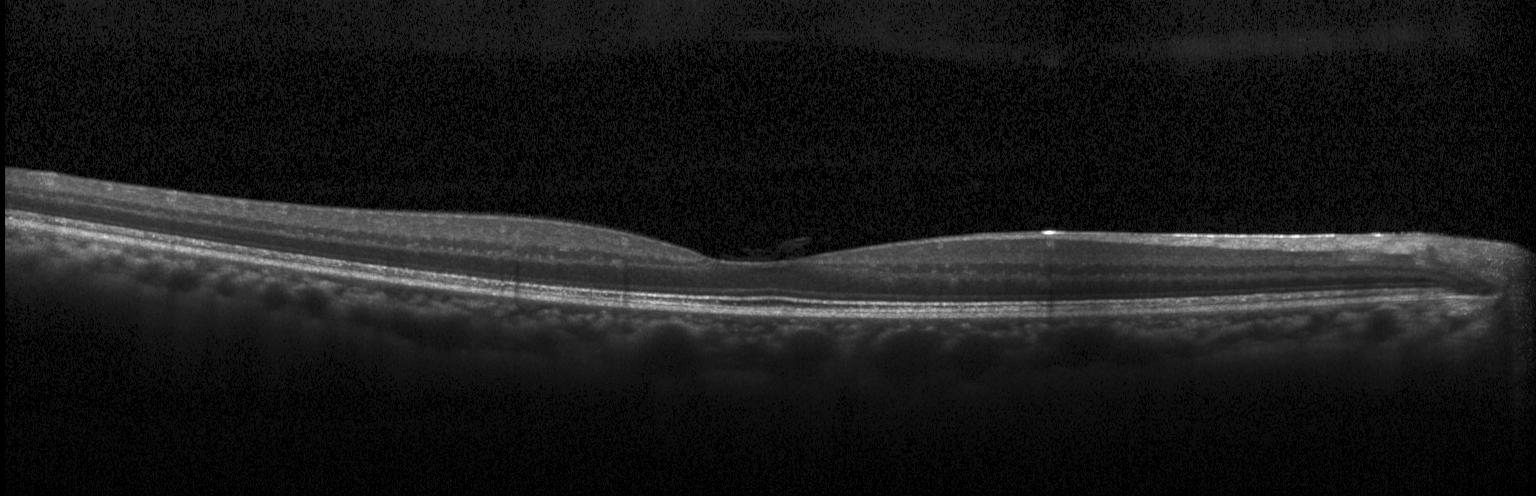 OCT B-scan. Through the macula
Impression: no evidence of choroidal neovascularization, diabetic macular edema, or drusen.